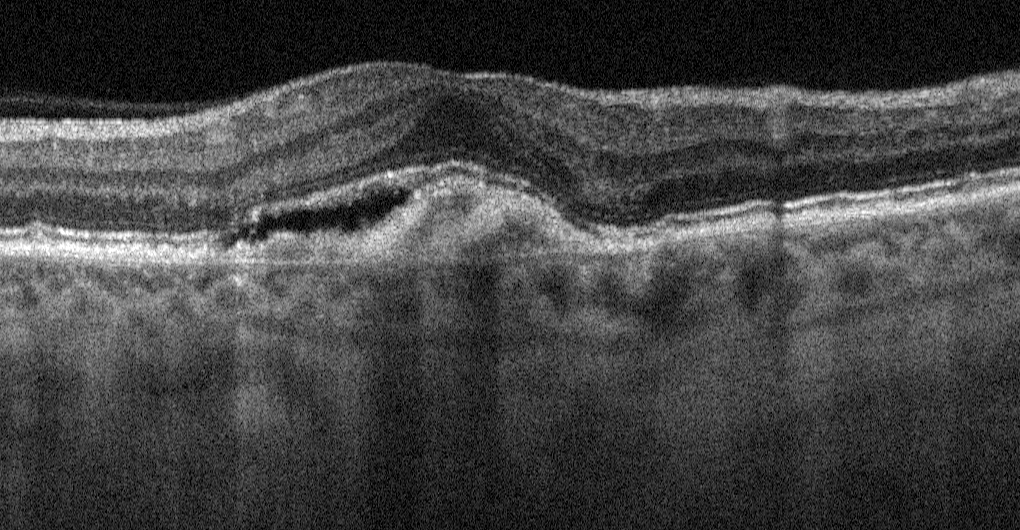

Macular OCT demonstrating age-related macular degeneration.